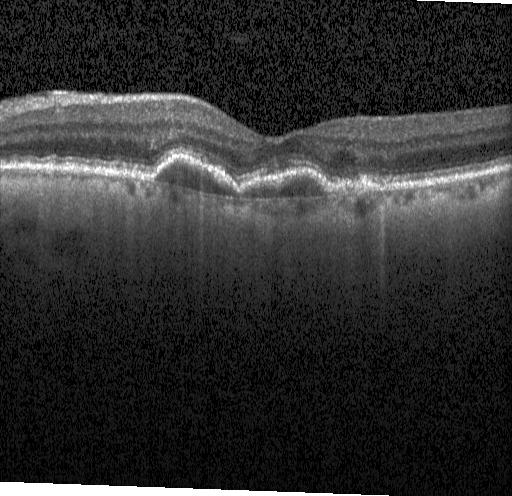 Heidelberg Spectralis OCT system. SD-OCT. Macular scan. Optical coherence tomography scan. Impression: a choroidal neovascular membrane.